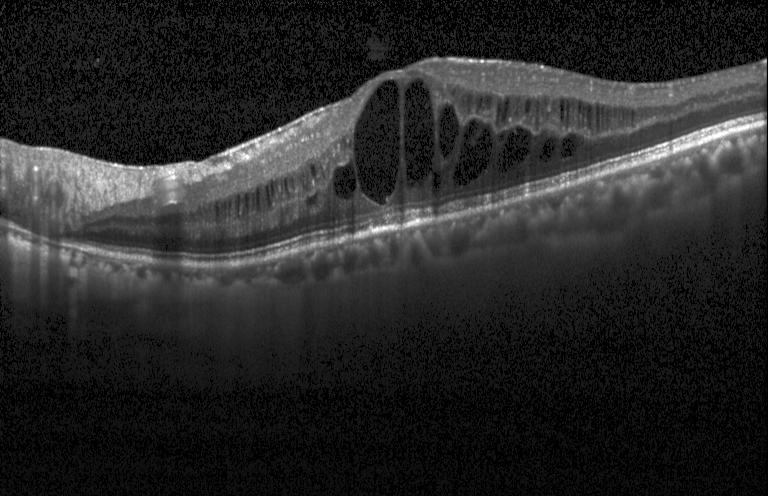
Horizontal scan through the fovea; SD-OCT; instrument: Heidelberg Spectralis; OCT B-scan
Impression: diabetic macular edema.